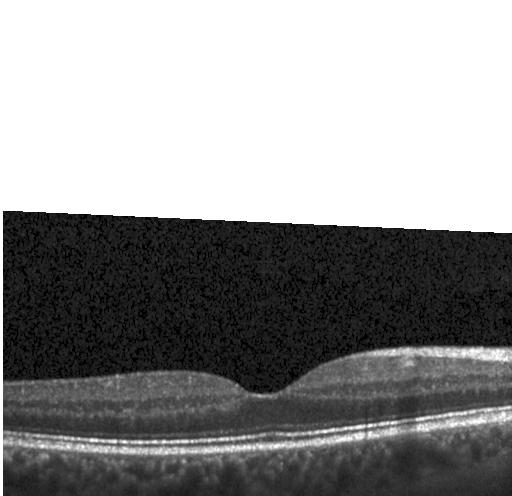
Optical coherence tomography B-scan. No choroidal neovascularization, no diabetic macular edema, and no drusen.